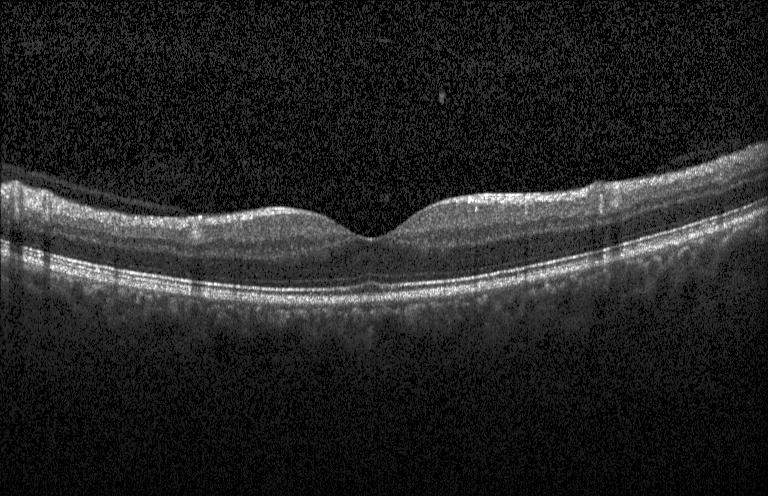 Heidelberg Spectralis OCT system. OCT B-scan. SD-OCT.
Assessment: no choroidal neovascularization, no diabetic macular edema, and no drusen.